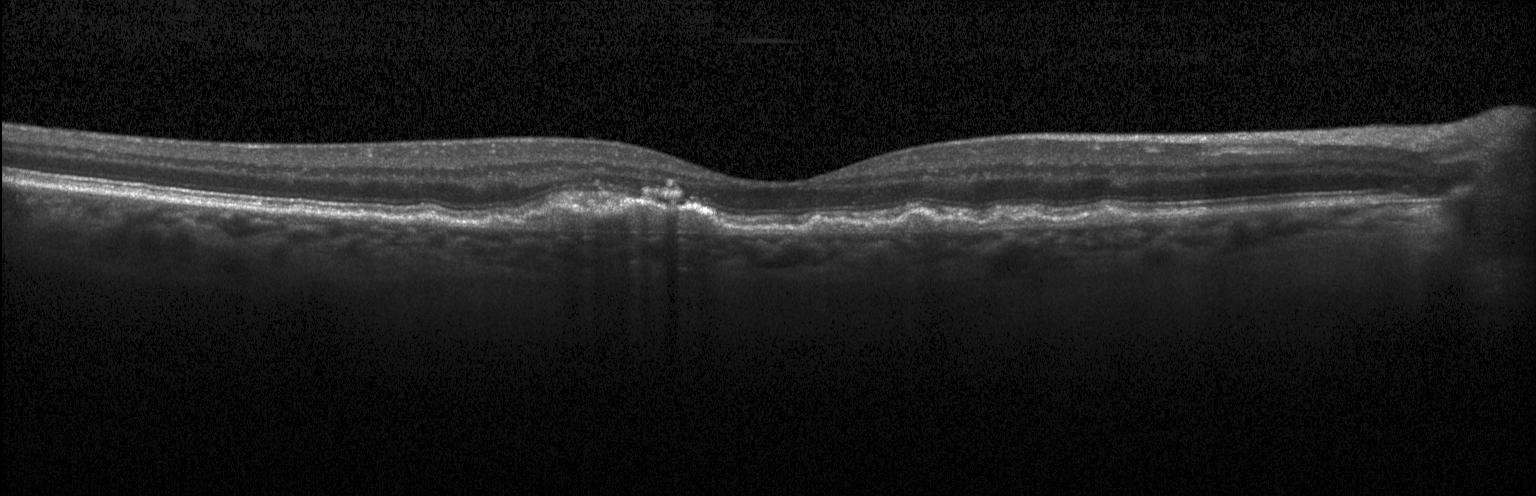
Finding: a choroidal neovascular membrane.